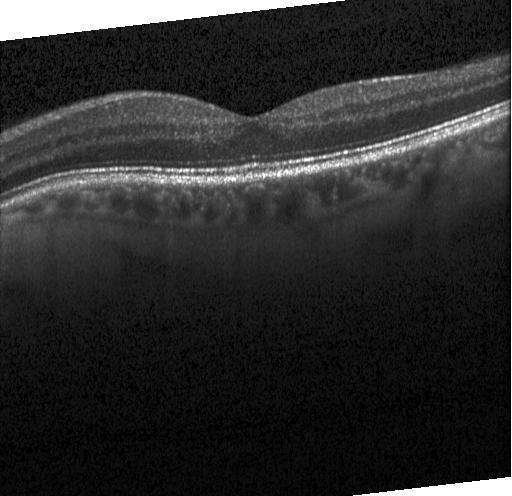
Macular OCT: no choroidal neovascularization, no diabetic macular edema, and no drusen.